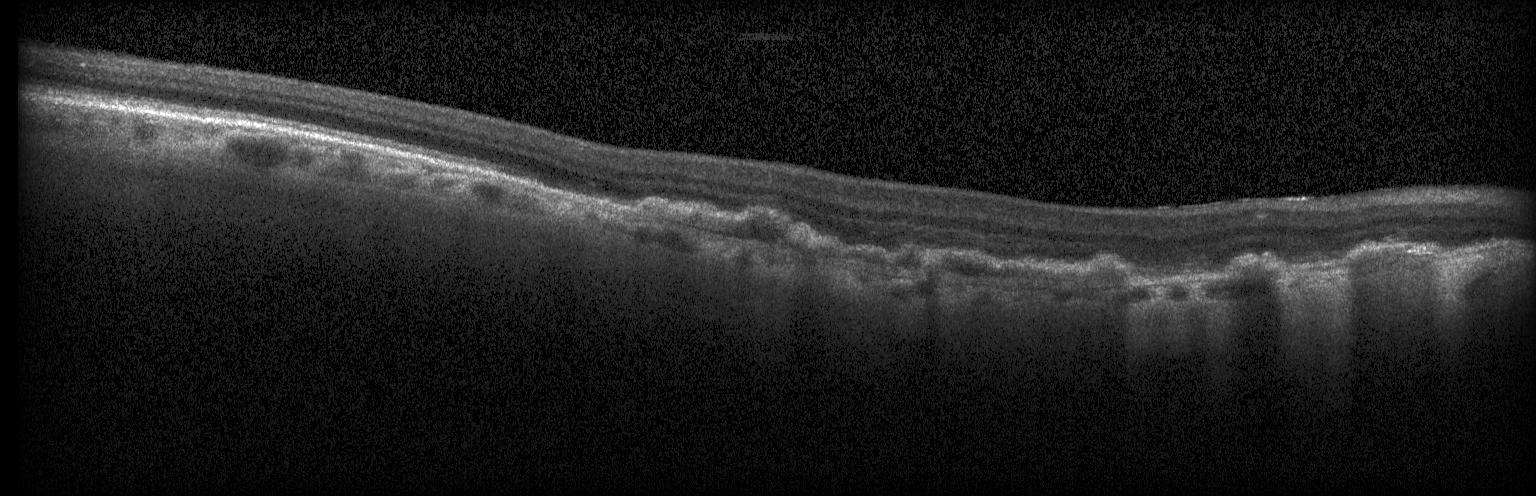 Assessment: a choroidal neovascular membrane.